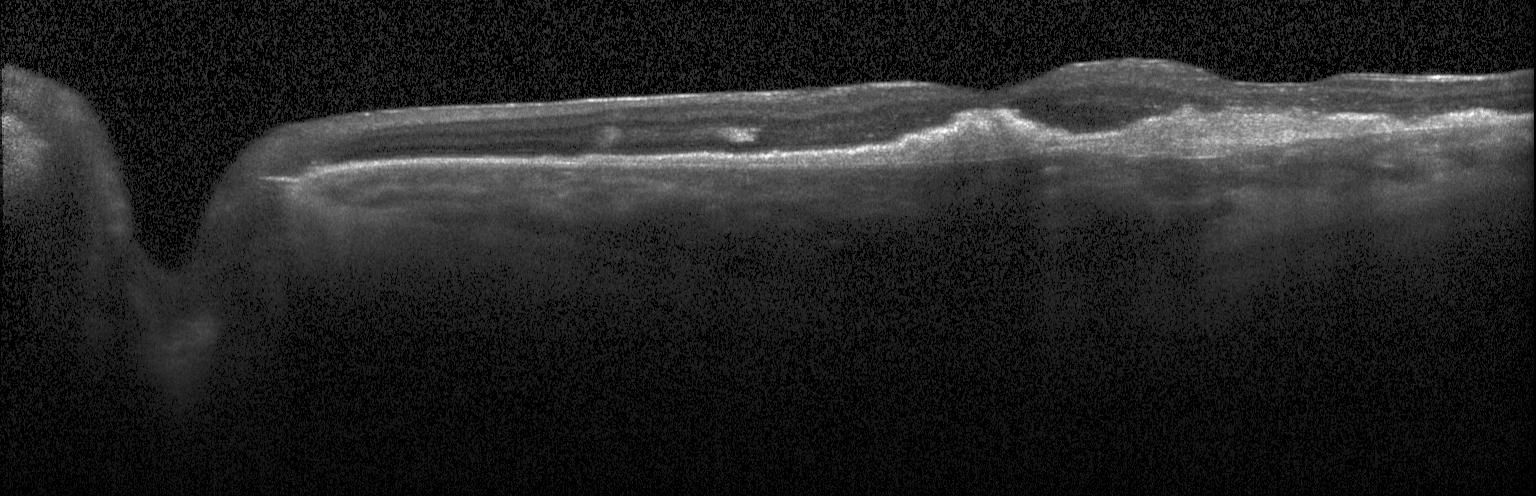

A choroidal neovascular membrane.